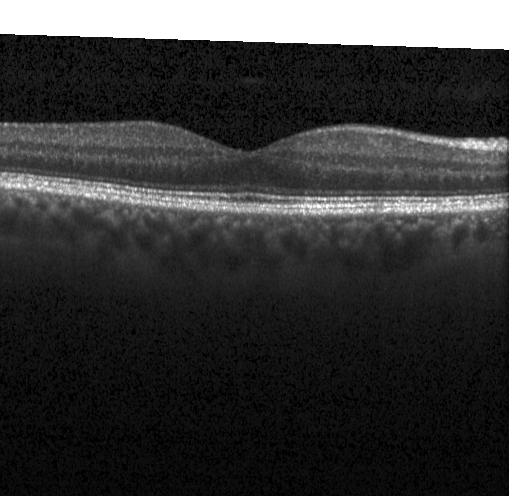
Finding: no choroidal neovascularization, no diabetic macular edema, and no drusen.